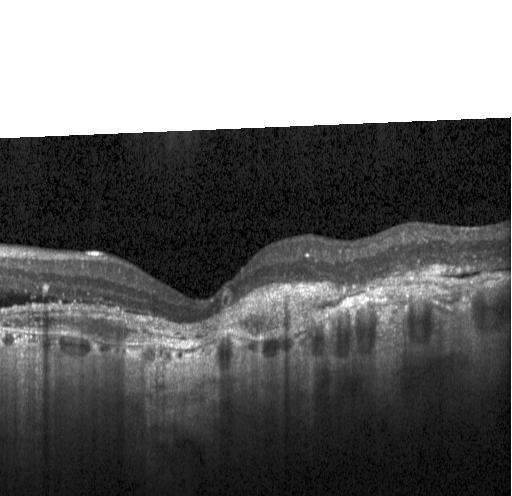
Optical coherence tomography scan · macular scan.
Impression: a choroidal neovascular membrane.